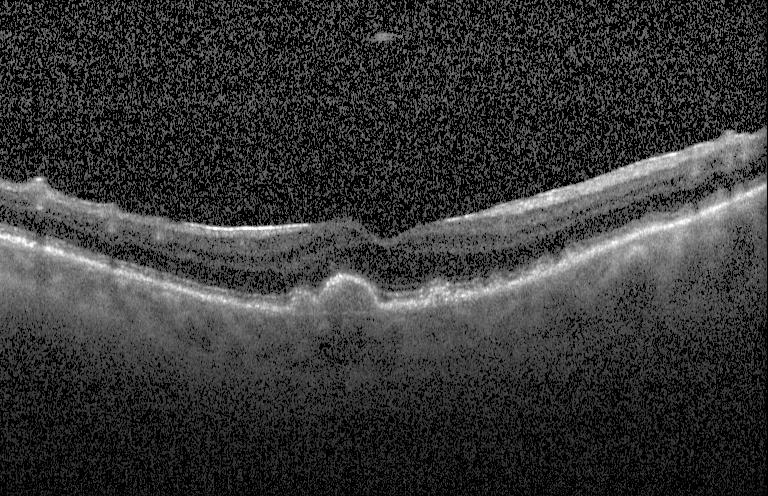
Sub-RPE drusenoid deposits.